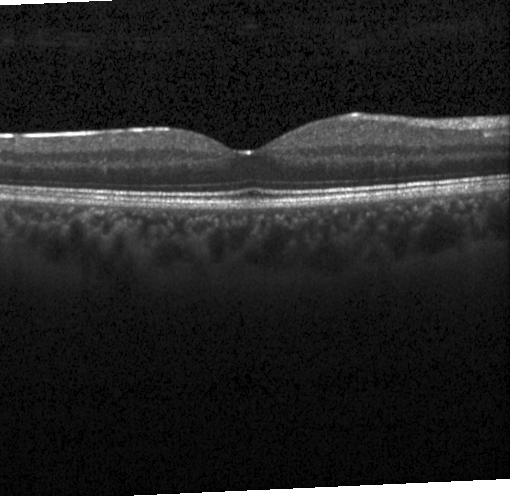

OCT B-scan. Spectral-domain optical coherence tomography. Instrument: Heidelberg Spectralis — Finding: no choroidal neovascularization, diabetic macular edema, or drusen.